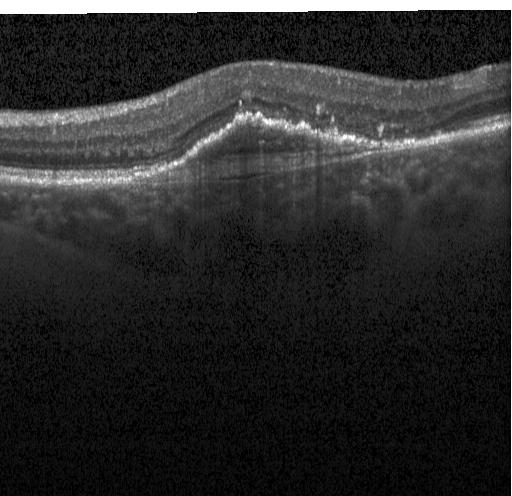

OCT scan showing a choroidal neovascular membrane.